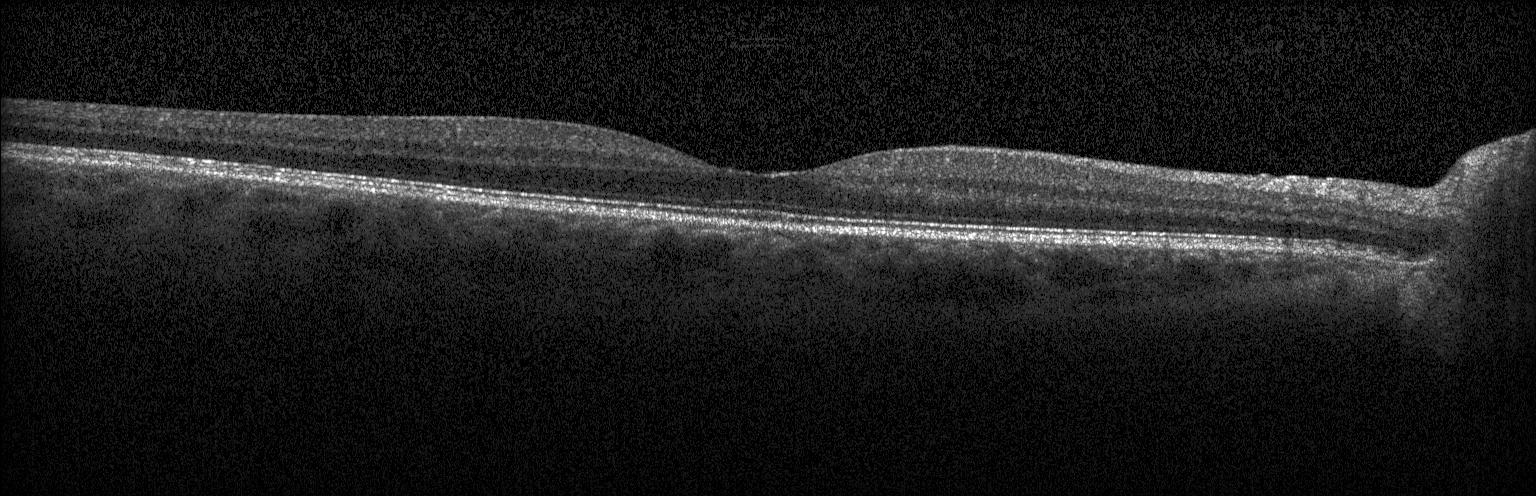
Diagnosis: no choroidal neovascularization, diabetic macular edema, or drusen.